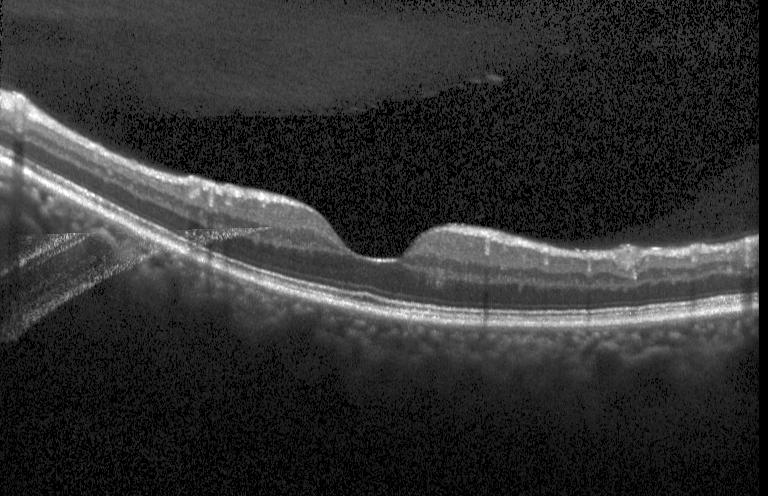
Retinal OCT B-scan. Dx: neither CNV, DME, nor drusen.